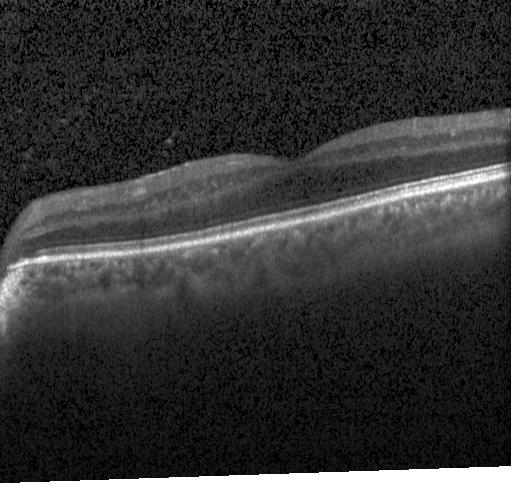

Retinal OCT cross-section — The scan shows no choroidal neovascularization, diabetic macular edema, or drusen.